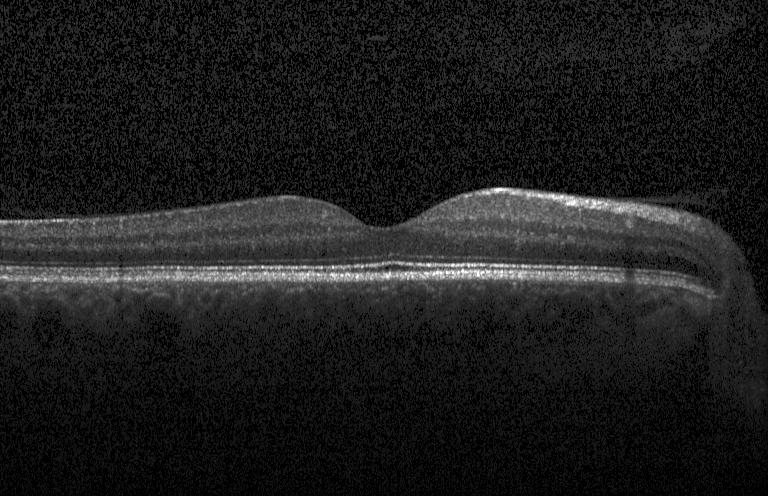 Dx: no choroidal neovascularization, no diabetic macular edema, and no drusen.